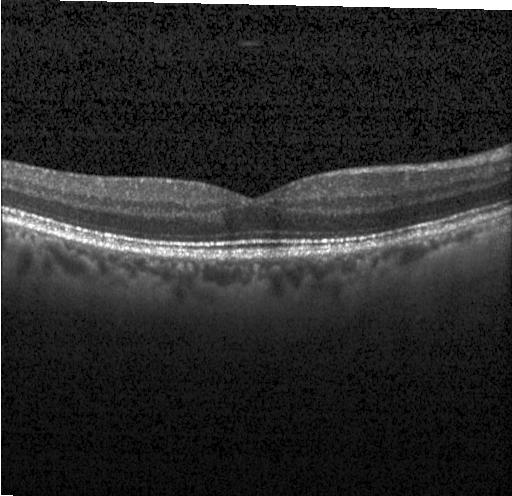

Finding: no evidence of choroidal neovascularization, diabetic macular edema, or drusen.